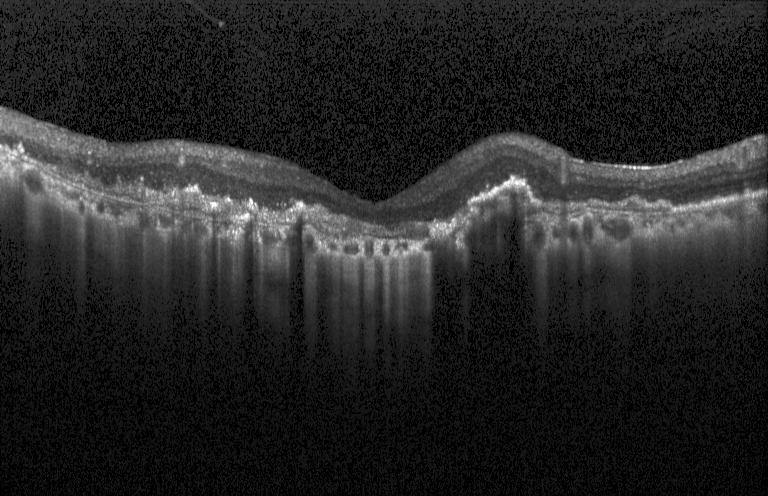 Optical coherence tomography B-scan
This B-scan demonstrates a choroidal neovascular membrane.